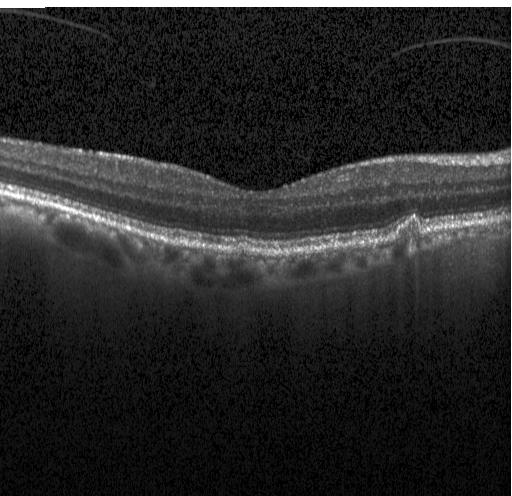

Optical coherence tomography B-scan. Impression: multiple drusen.